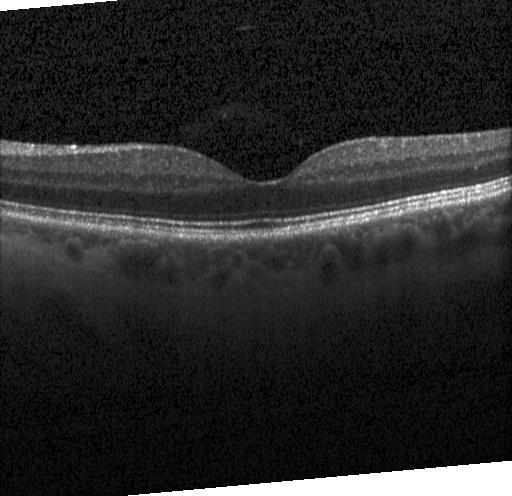 OCT line scan; macular scan; spectral-domain OCT.
Diagnosis: no choroidal neovascularization, diabetic macular edema, or drusen.